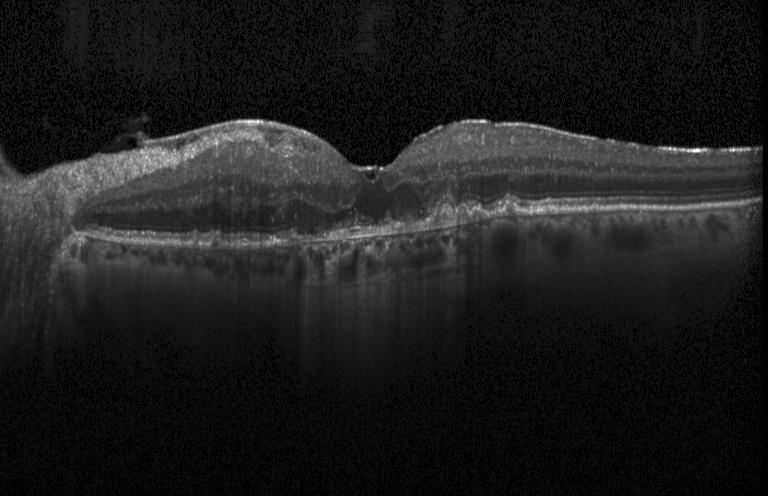 Impression: choroidal neovascularization.